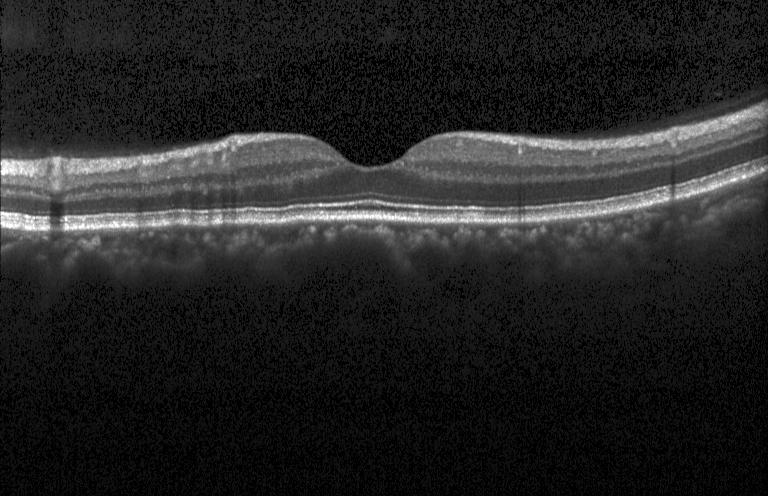
Diagnosis: no CNV, no DME, and no drusen.